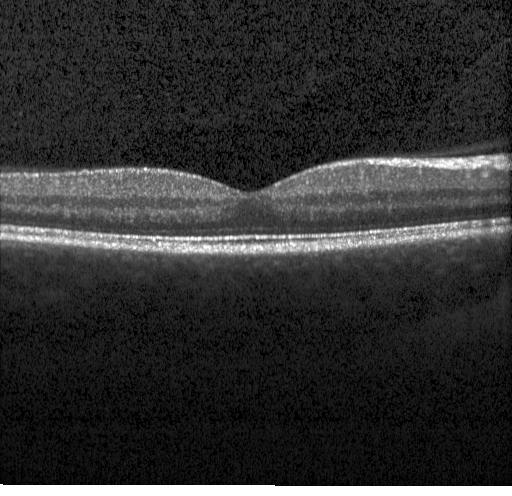
Macular scan, Heidelberg Spectralis OCT system, spectral-domain OCT, retinal OCT B-scan. Assessment: no CNV, no DME, and no drusen.